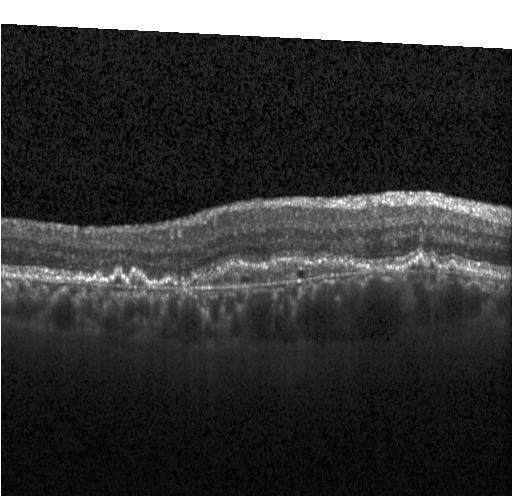 Through the macula, optical coherence tomography scan, instrument: Heidelberg Spectralis — Finding: a choroidal neovascular membrane.